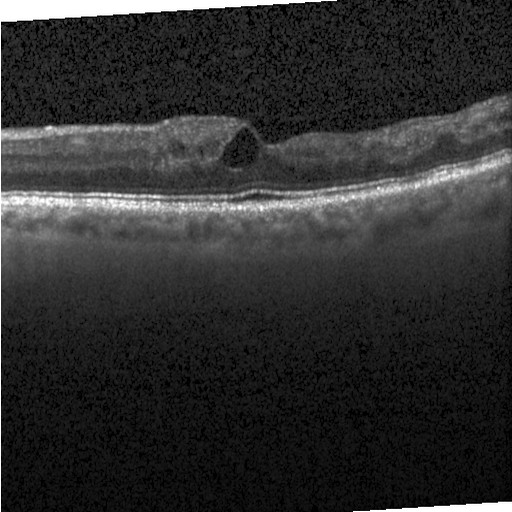
Diagnosis: diabetic macular edema.